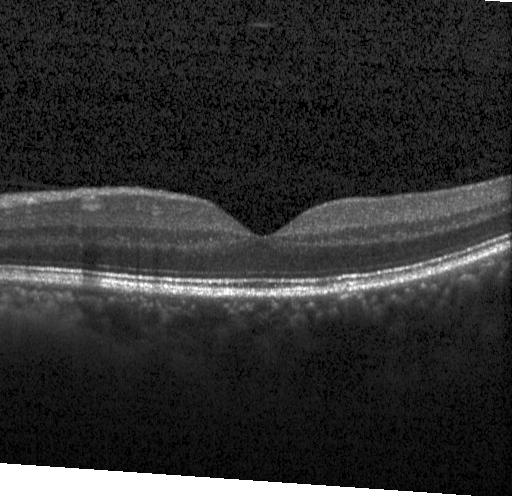

Instrument: Heidelberg Spectralis; optical coherence tomography B-scan
Neither CNV, DME, nor drusen.